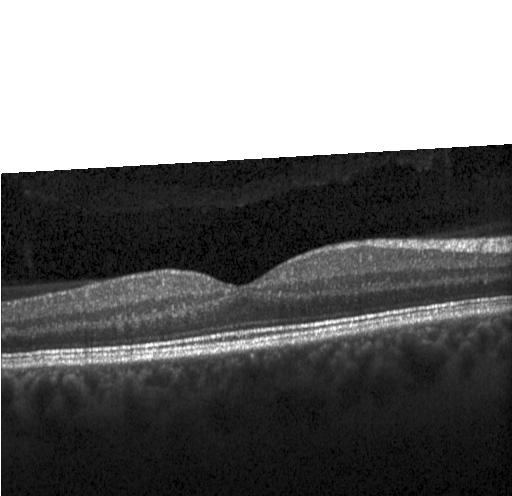
Impression: neither choroidal neovascularization, diabetic macular edema, nor drusen.